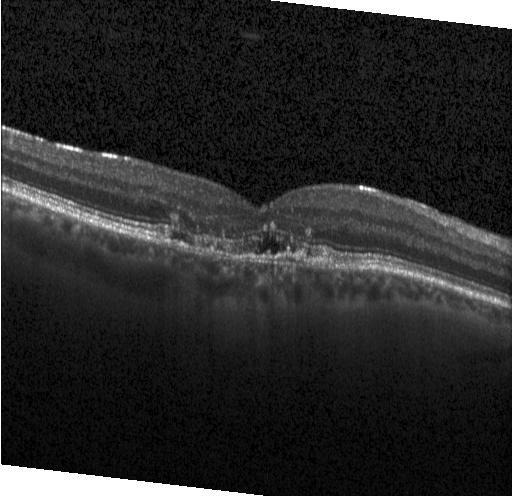
Diagnosis: choroidal neovascularization.